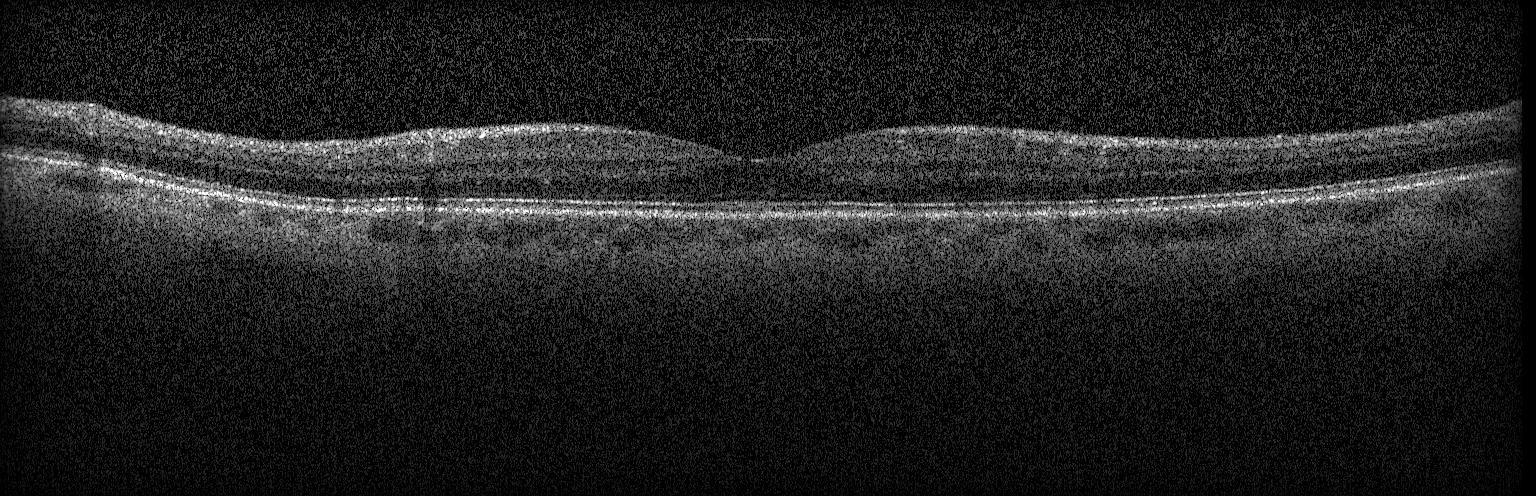
This B-scan demonstrates no choroidal neovascularization, no diabetic macular edema, and no drusen.